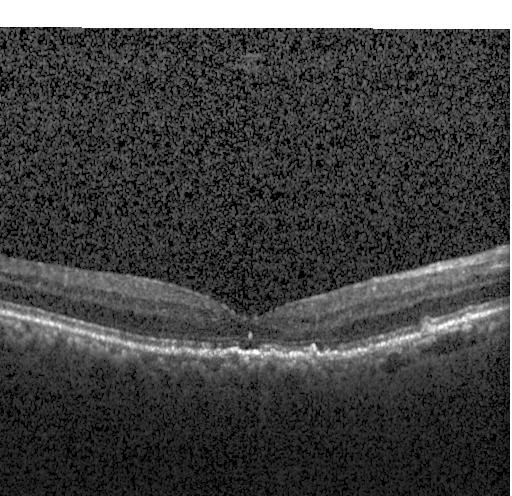 Spectral-domain OCT; Heidelberg Spectralis OCT system; optical coherence tomography B-scan; centered on the fovea — Finding: multiple drusen.